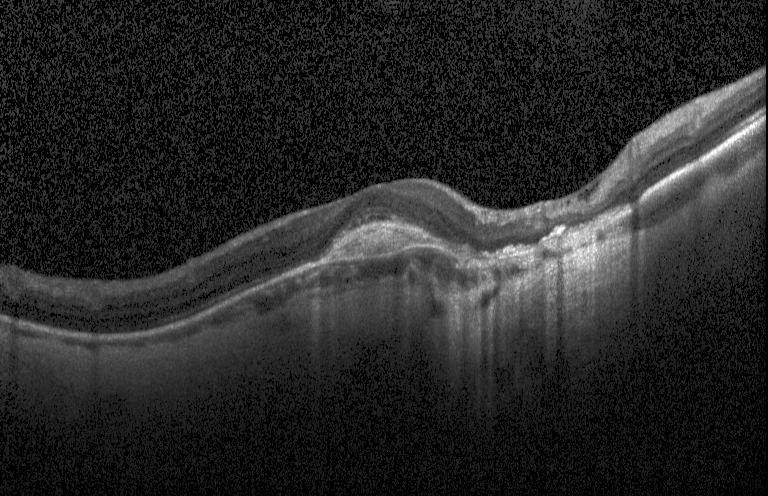 This B-scan demonstrates a choroidal neovascular membrane.